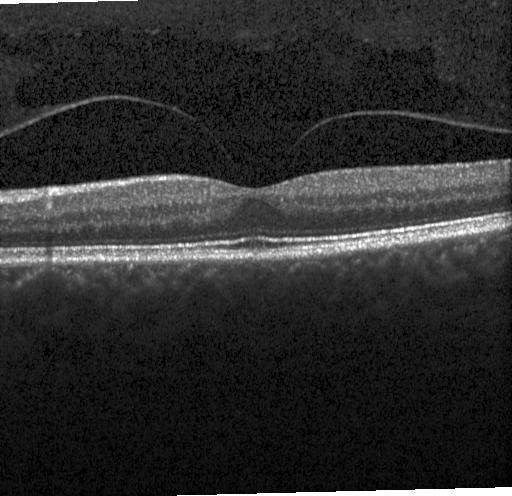
Retinal OCT cross-section; spectral-domain OCT; acquired on a Heidelberg Spectralis; horizontal scan through the fovea — Diagnosis: no choroidal neovascularization, diabetic macular edema, or drusen.